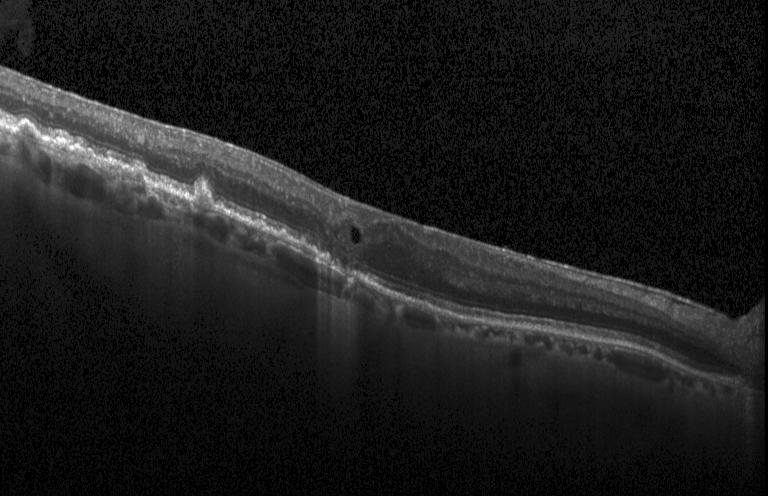

Impression: choroidal neovascularization (CNV).